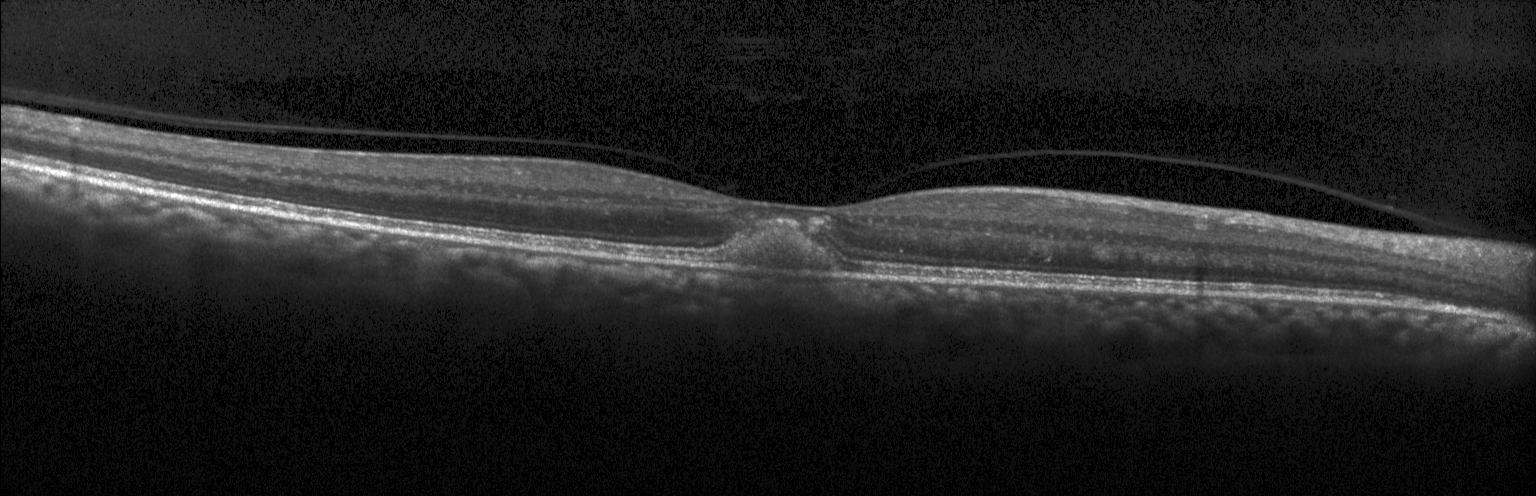
OCT line scan.
Diagnosis: choroidal neovascularization (CNV).